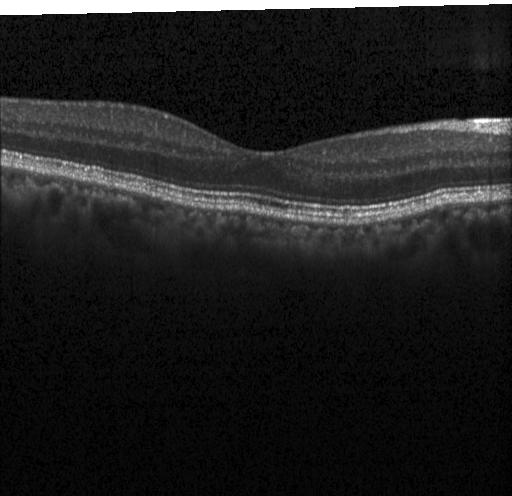 OCT line scan
Diagnosis: no choroidal neovascularization, no diabetic macular edema, and no drusen.